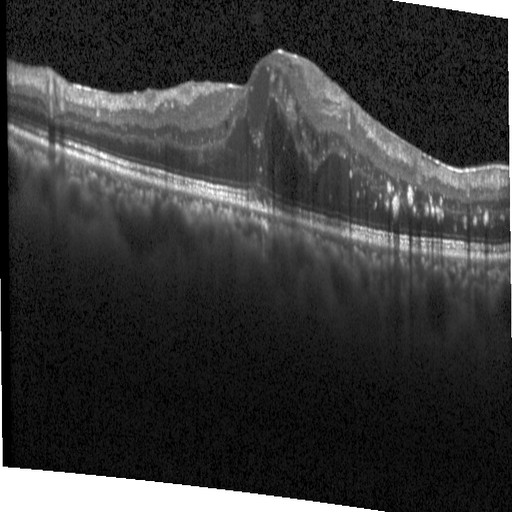 OCT B-scan.
Finding: diabetic macular edema.